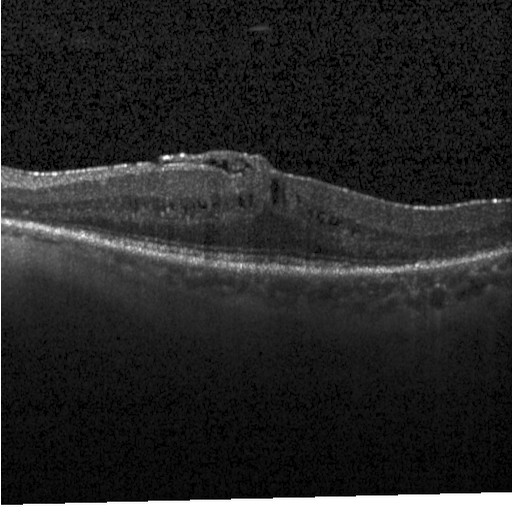

The scan shows diabetic macular edema.